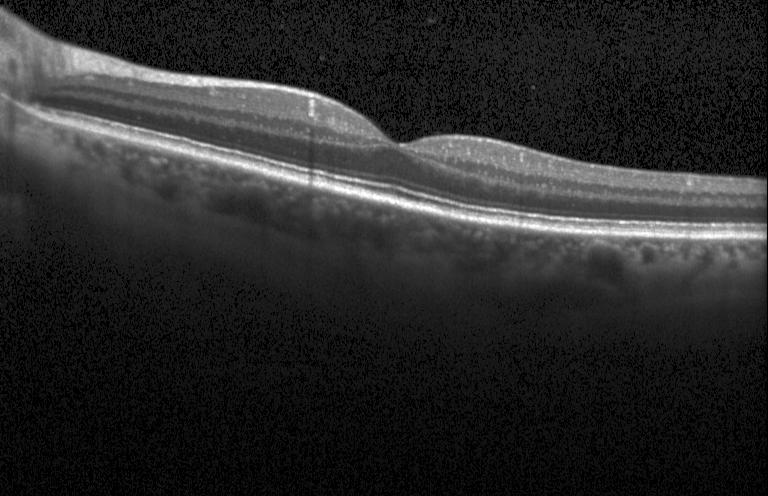
OCT B-scan. Spectral-domain optical coherence tomography
Macular OCT: no choroidal neovascularization, no diabetic macular edema, and no drusen.